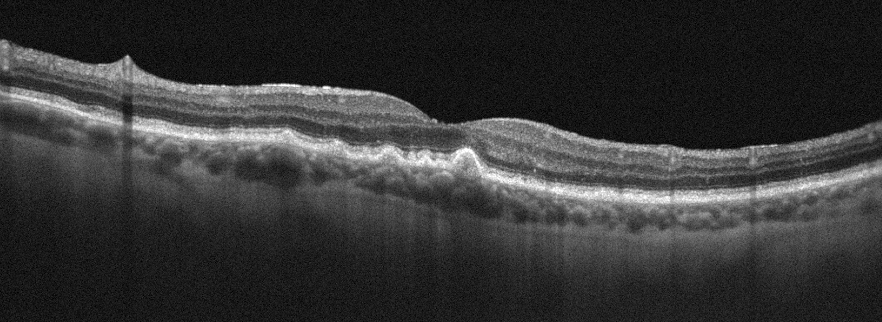 Optical coherence tomography B-scan · OD — Macular OCT: age-related macular degeneration.